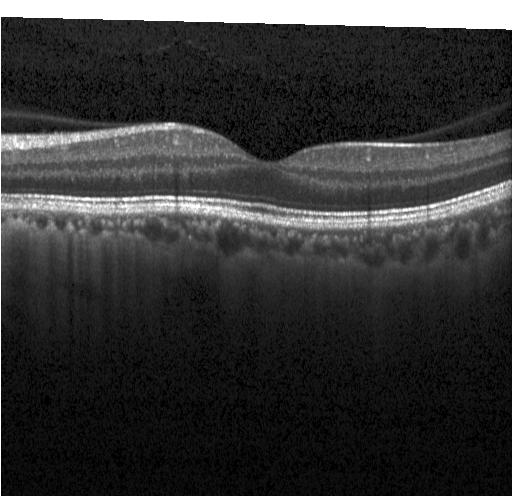
Horizontal scan through the fovea. Optical coherence tomography B-scan. SD-OCT. Heidelberg Spectralis OCT system — Diagnosis: no choroidal neovascularization, diabetic macular edema, or drusen.